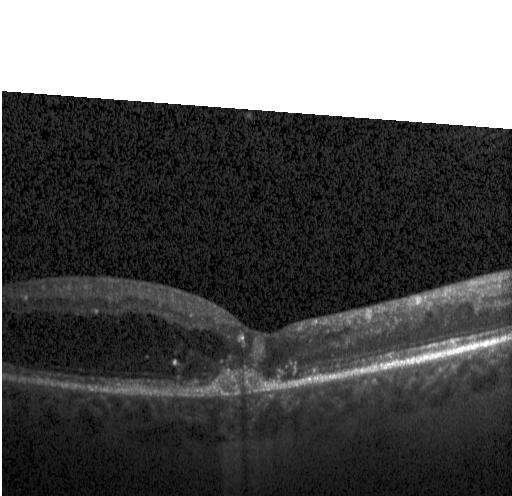

Macular OCT demonstrating diabetic macular edema.